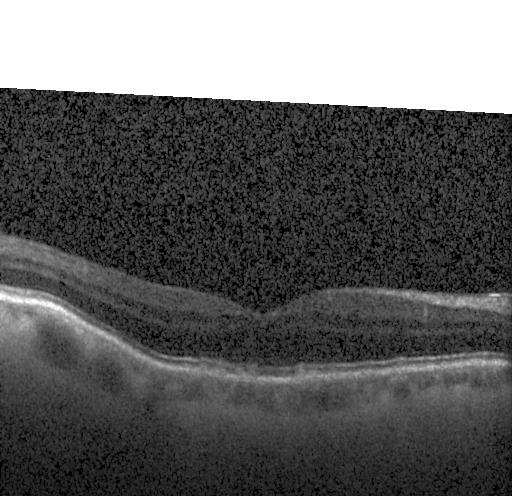
OCT line scan, Heidelberg Spectralis — Impression: multiple drusen.